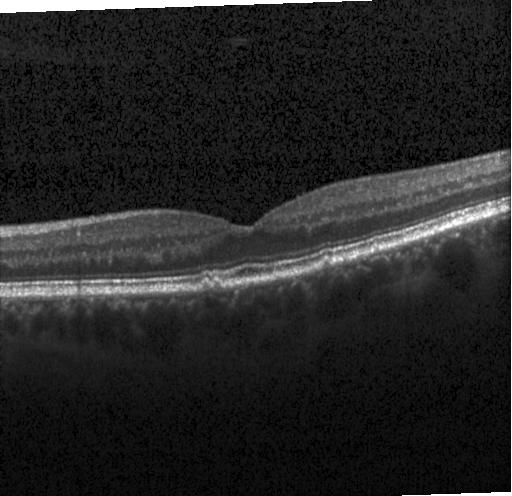 Impression: sub-RPE drusenoid deposits.